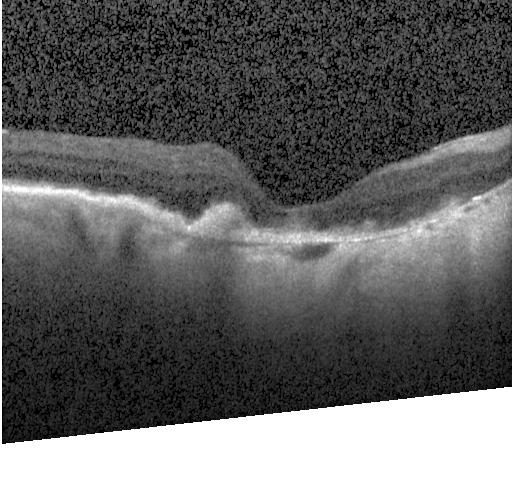

Spectral-domain optical coherence tomography, optical coherence tomography B-scan — Macular OCT: a choroidal neovascular membrane.